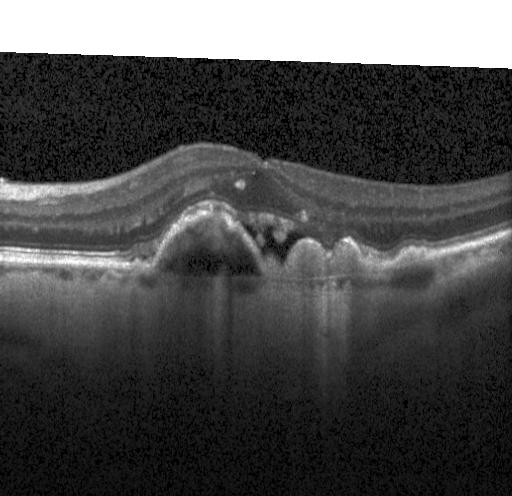
Assessment: choroidal neovascularization (CNV).